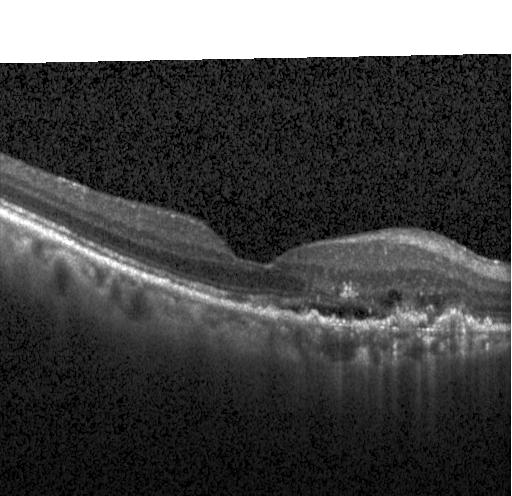 The scan shows choroidal neovascularization (CNV).